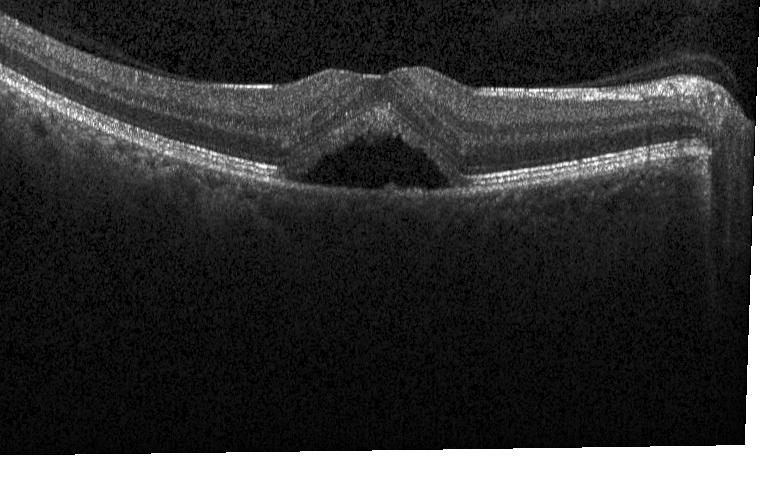

Dx: choroidal neovascularization (CNV).